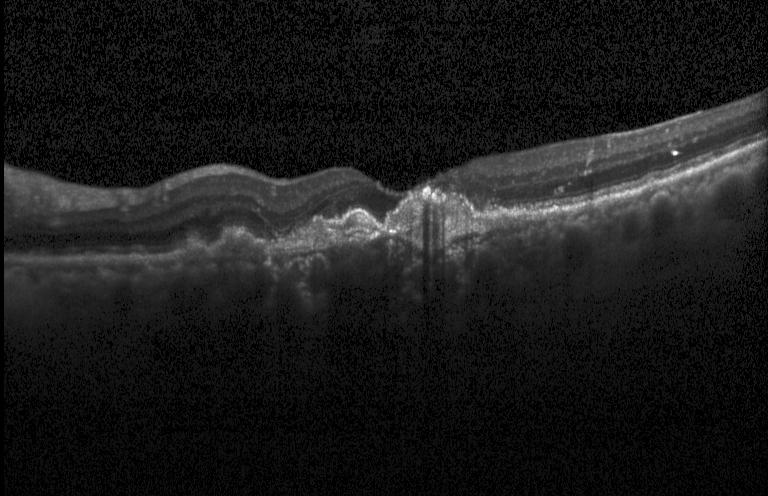
Diagnosis: a choroidal neovascular membrane.